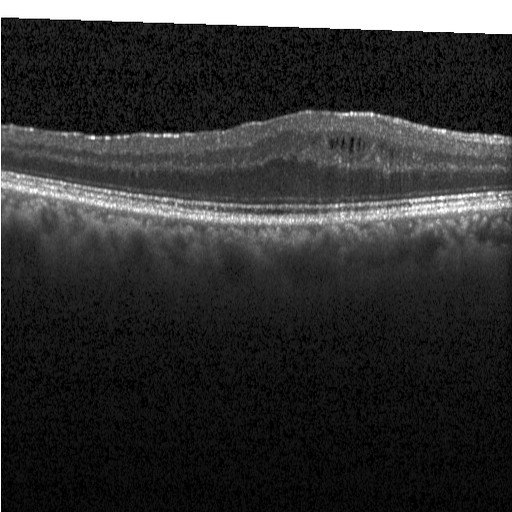 Impression: DME.